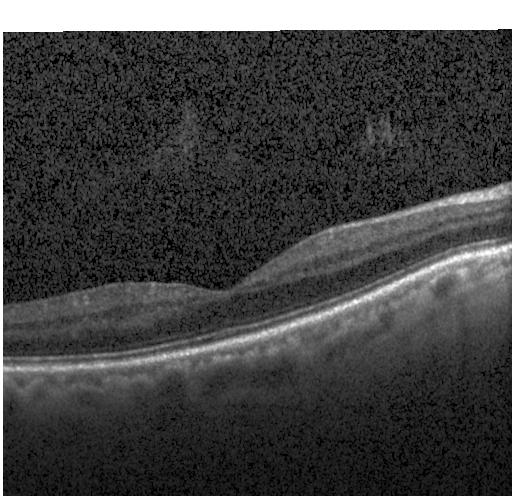 Optical coherence tomography scan — Diagnosis: no evidence of choroidal neovascularization, diabetic macular edema, or drusen.